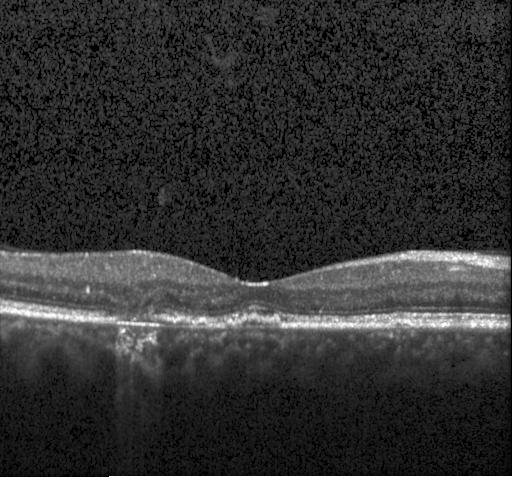

Retinal OCT B-scan. Heidelberg Spectralis
Diagnosis: choroidal neovascularization.